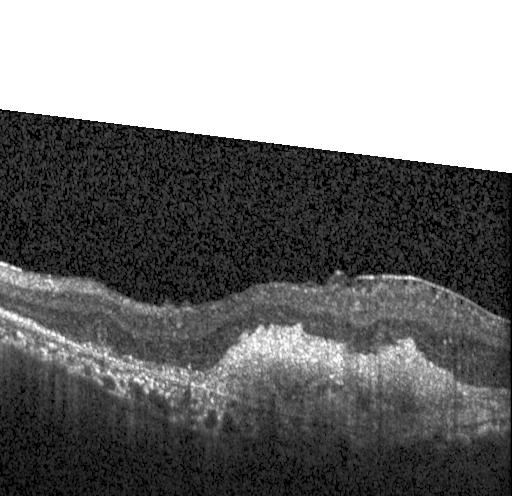

This B-scan demonstrates a choroidal neovascular membrane.